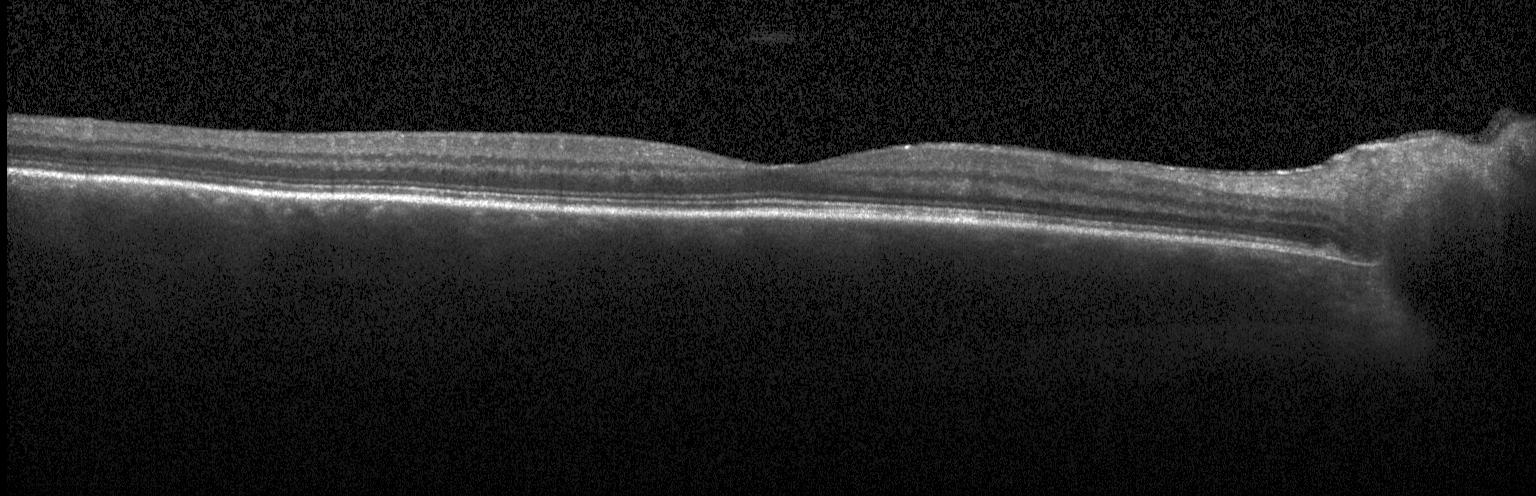 OCT line scan — Diagnosis: no evidence of choroidal neovascularization, diabetic macular edema, or drusen.